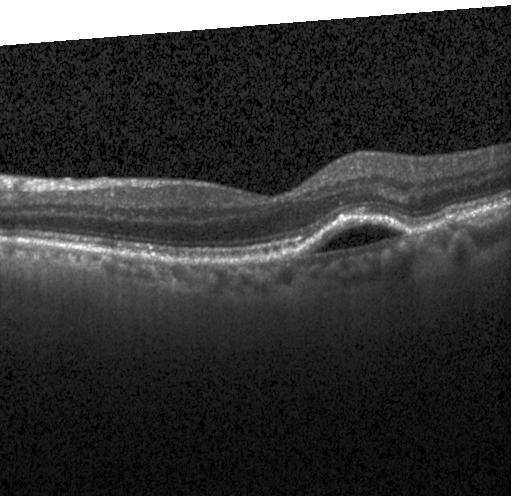
Macular OCT demonstrating a choroidal neovascular membrane.